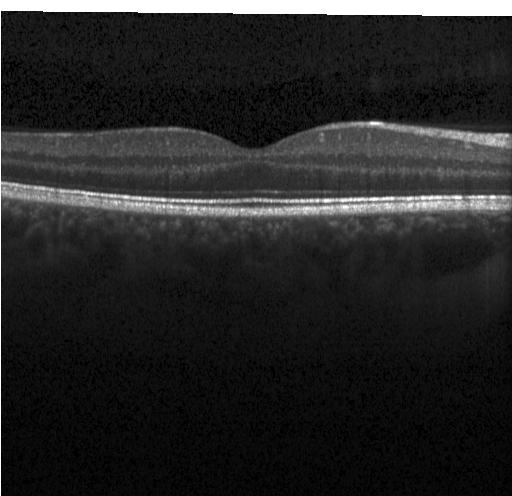

Optical coherence tomography B-scan
Impression: no evidence of CNV, DME, or drusen.